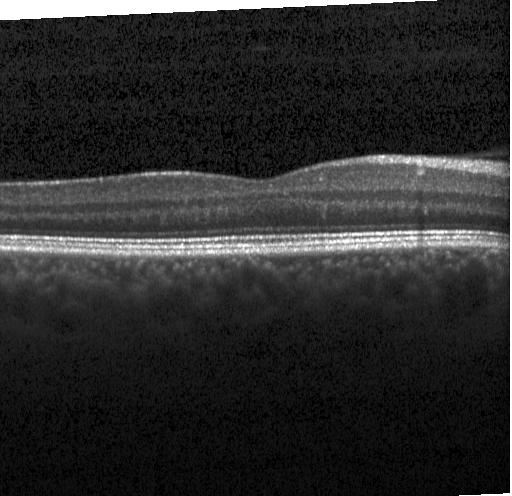
Optical coherence tomography B-scan. This B-scan demonstrates no evidence of CNV, DME, or drusen.